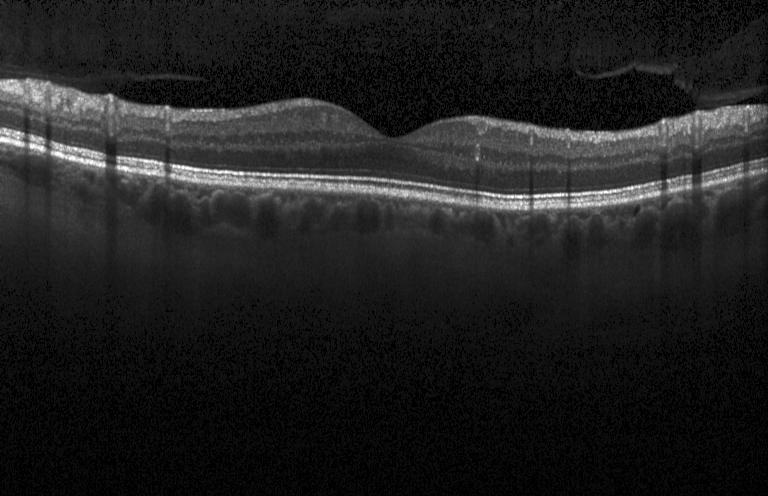
This B-scan demonstrates no choroidal neovascularization, no diabetic macular edema, and no drusen.